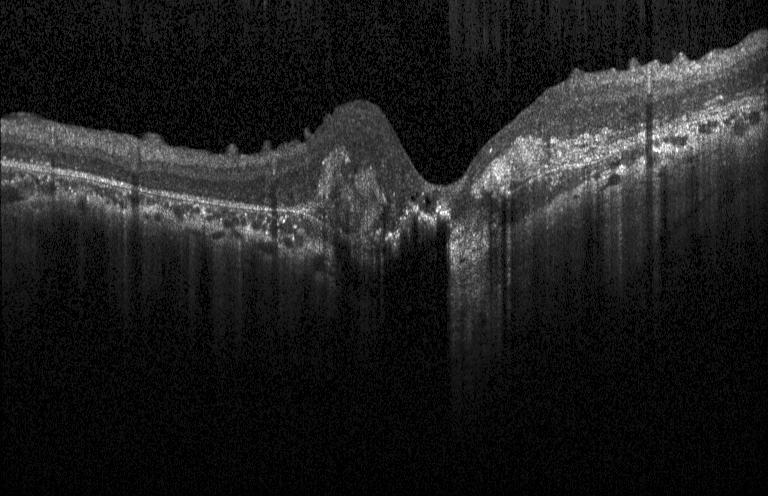
OCT B-scan showing a choroidal neovascular membrane.